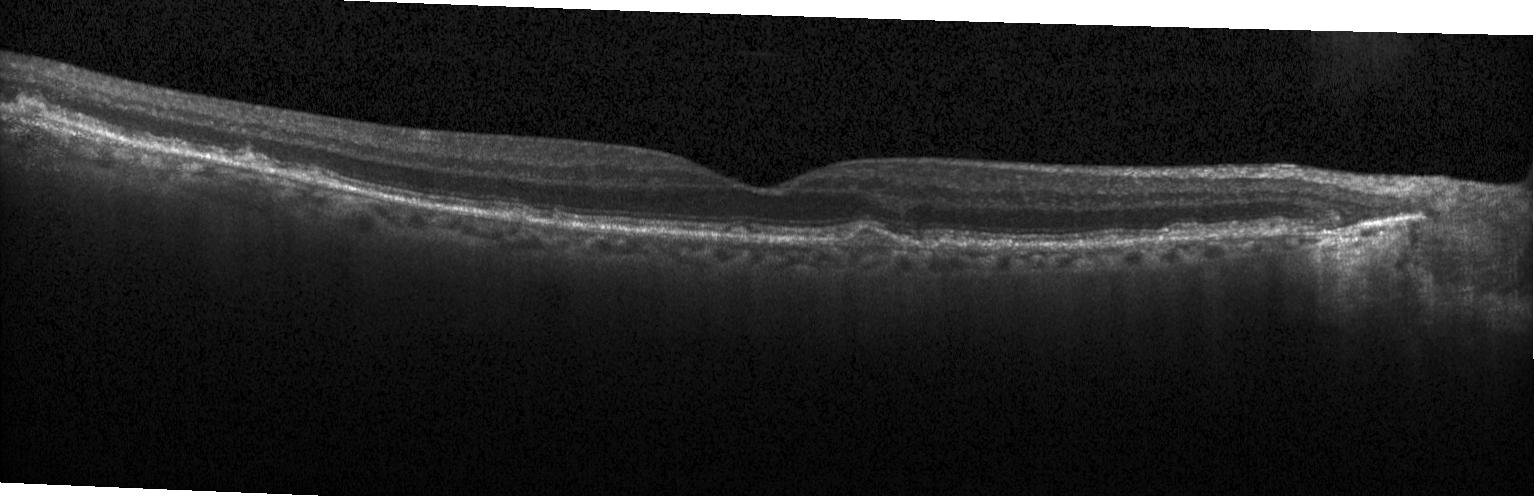

Acquired on a Heidelberg Spectralis · spectral-domain optical coherence tomography · optical coherence tomography B-scan · macular scan. Dx: sub-RPE drusenoid deposits.